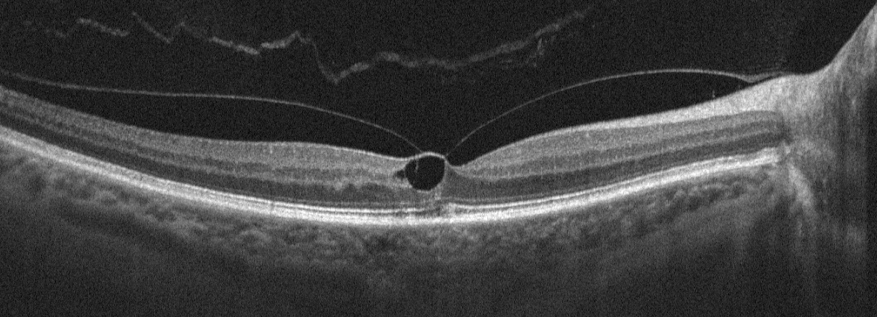 Retinal OCT cross-section
Macular OCT: vitreomacular interface disease.